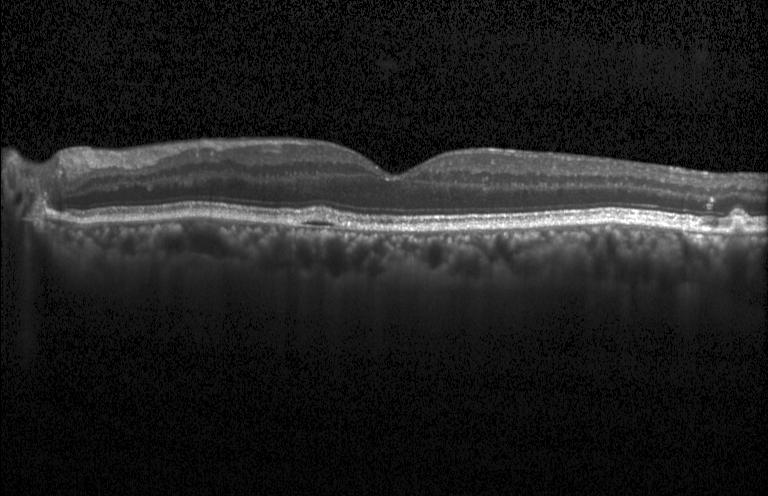 Impression: multiple drusen.